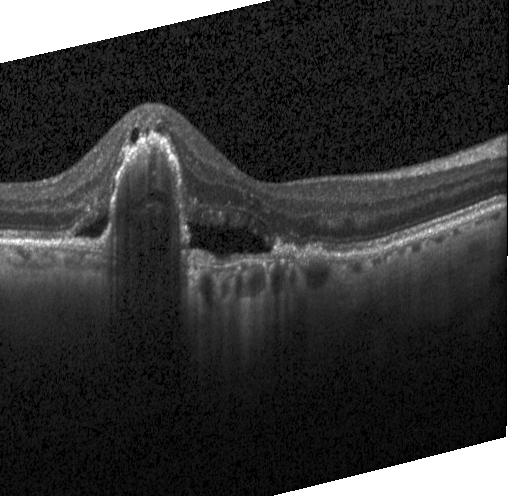
Retinal OCT B-scan; macular scan
Impression: a choroidal neovascular membrane.